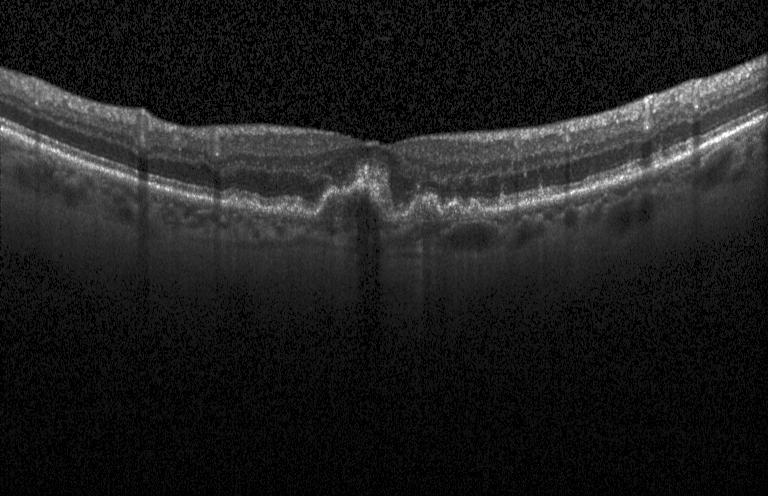
Through the macula. Optical coherence tomography B-scan. Assessment: a choroidal neovascular membrane.